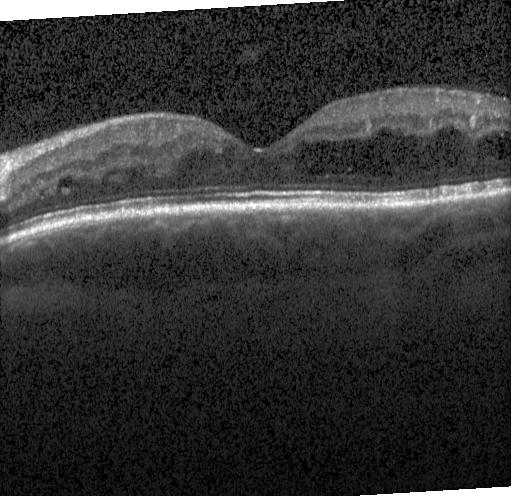

Retinal OCT cross-section; Heidelberg Spectralis; through the macula — This B-scan demonstrates diabetic macular edema.